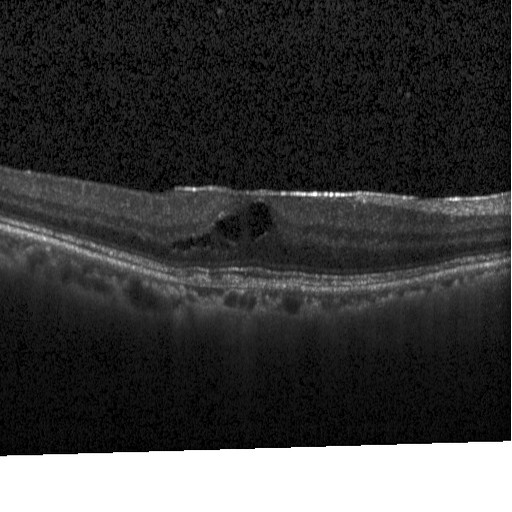 Spectral-domain optical coherence tomography. Acquired on a Heidelberg Spectralis. Optical coherence tomography scan. Finding: diabetic macular edema.